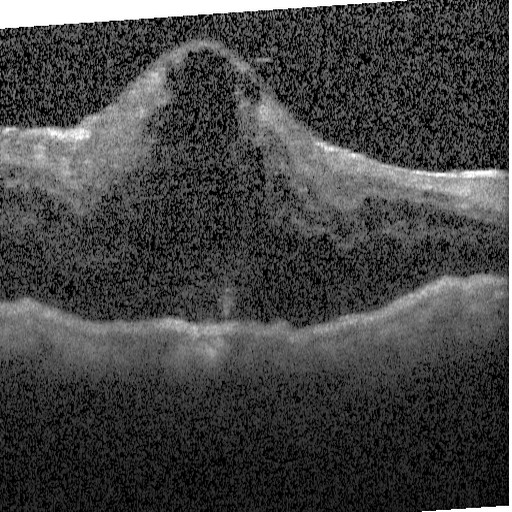
Diabetic macular edema (DME).